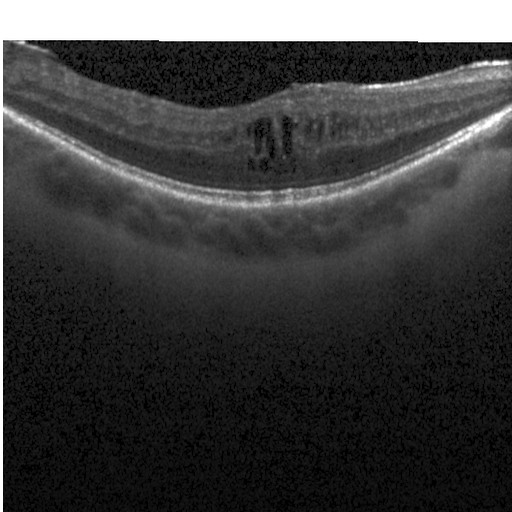

Diabetic macular edema.